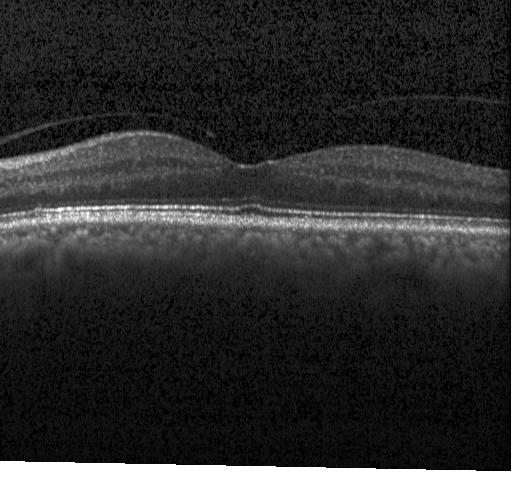 Macular OCT demonstrating neither CNV, DME, nor drusen.